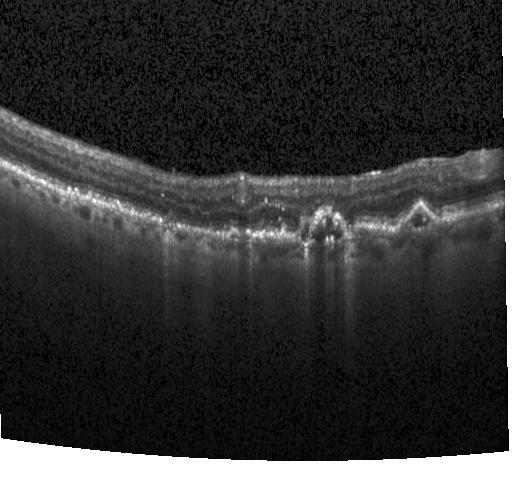 Instrument: Heidelberg Spectralis, OCT line scan, centered on the fovea. OCT finding: CNV.